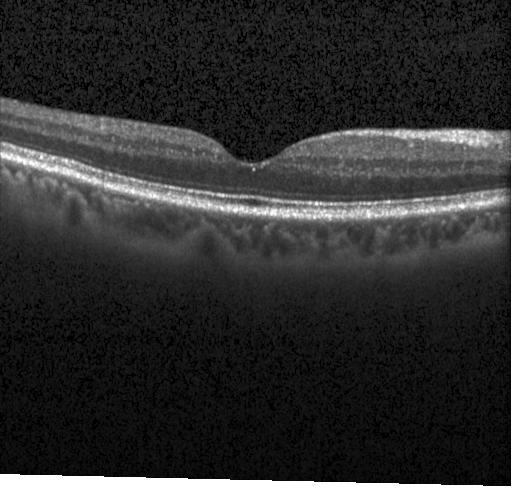
Through the macula, OCT B-scan, SD-OCT, Heidelberg Spectralis — Neither CNV, DME, nor drusen.